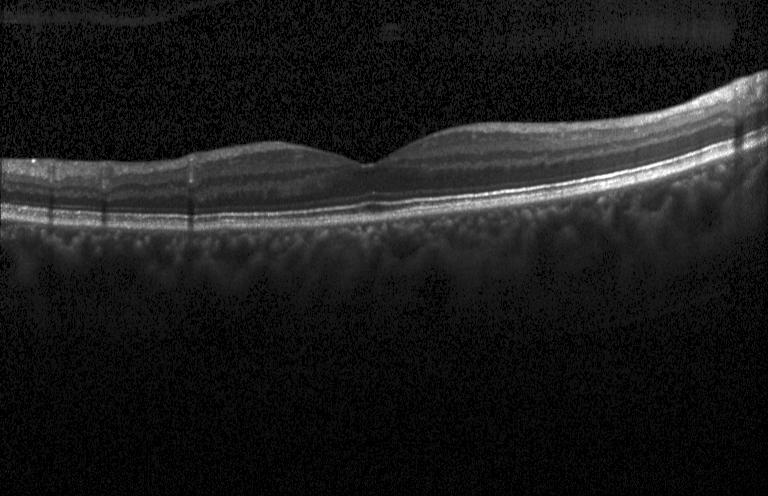 Horizontal scan through the fovea · acquired on a Heidelberg Spectralis · SD-OCT · retinal OCT B-scan. Macular OCT: no CNV, no DME, and no drusen.